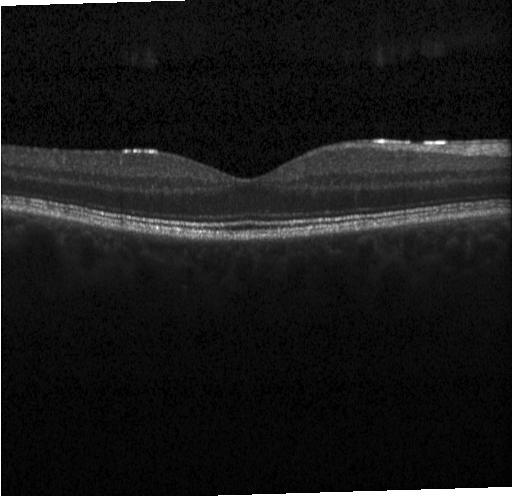
Macular OCT: no choroidal neovascularization, diabetic macular edema, or drusen.